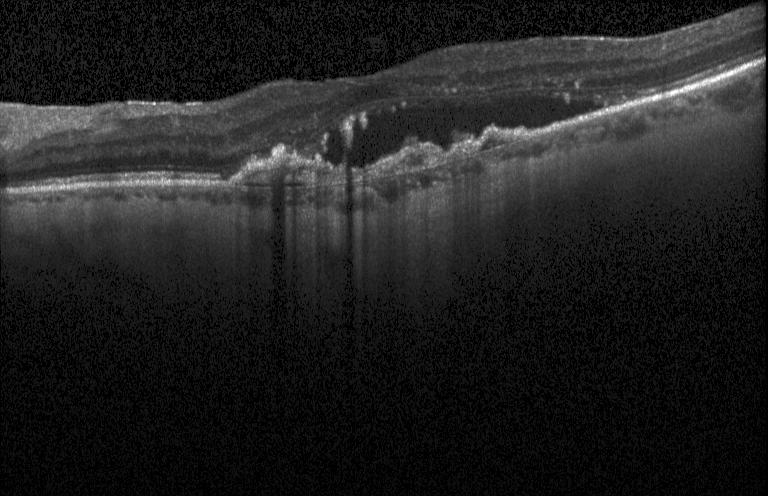

Heidelberg Spectralis OCT system · retinal OCT cross-section · fovea-centered.
Diagnosis: CNV.